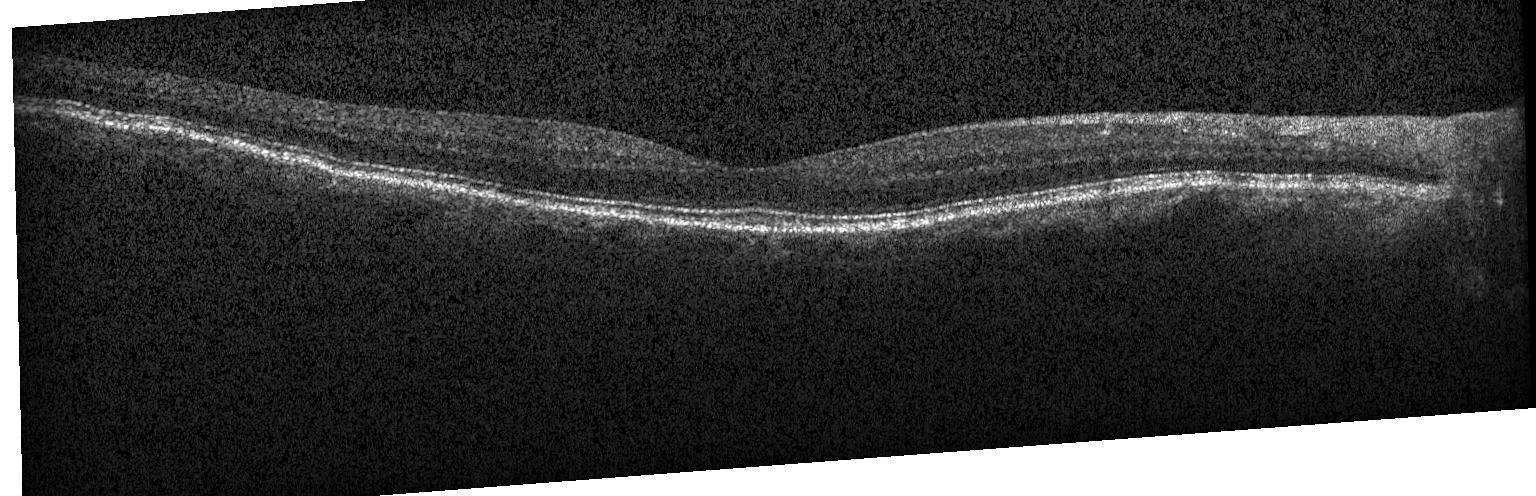
Finding: neither choroidal neovascularization, diabetic macular edema, nor drusen.